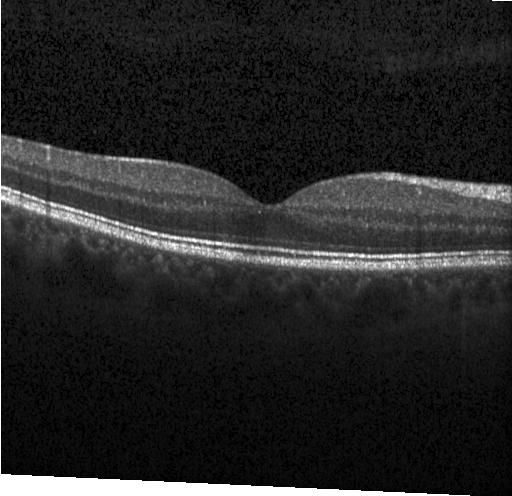
Macular OCT demonstrating no choroidal neovascularization, diabetic macular edema, or drusen.